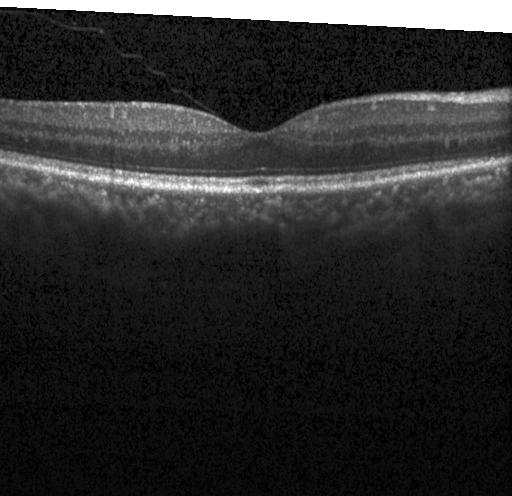

Retinal OCT cross-section showing no choroidal neovascularization, no diabetic macular edema, and no drusen.